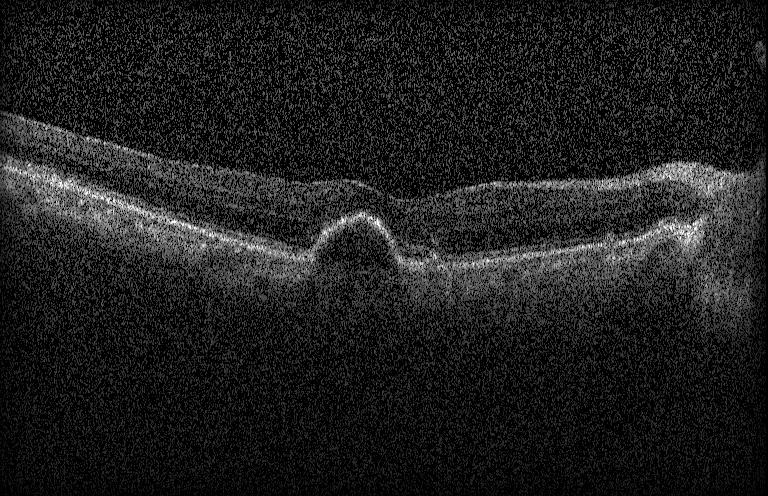 OCT finding: choroidal neovascularization.